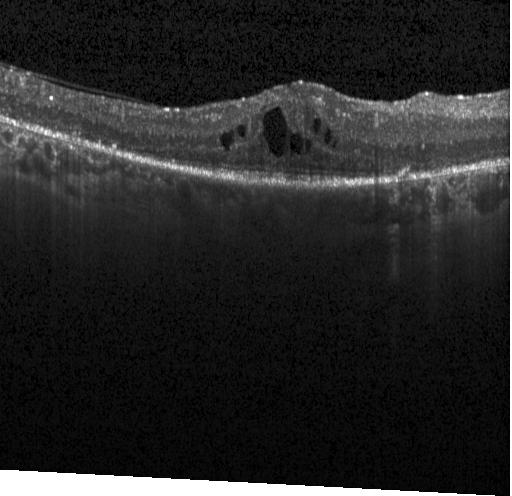
The scan shows diabetic macular edema (DME).